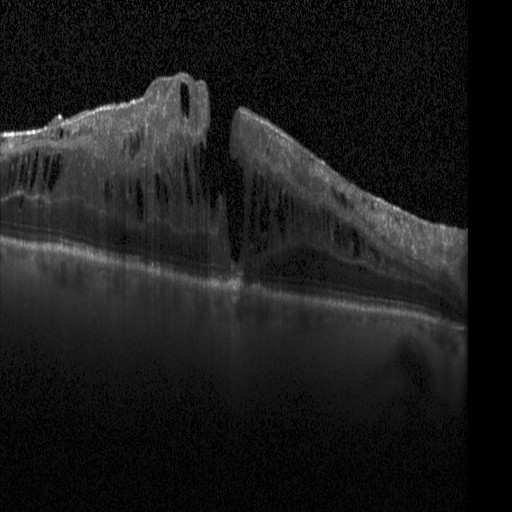

Heidelberg Spectralis OCT system · OCT B-scan · through the macula — The scan shows diabetic macular edema (DME).